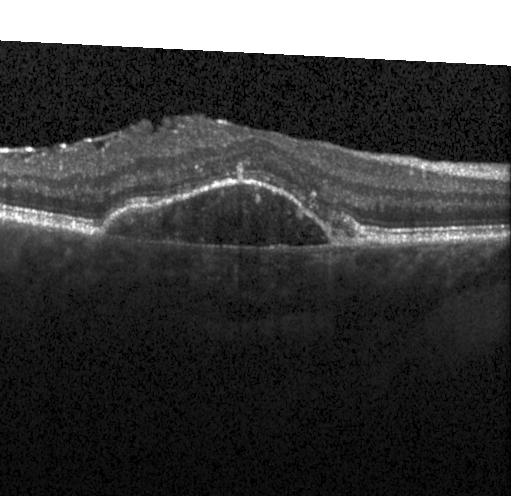
Heidelberg Spectralis OCT system. Optical coherence tomography scan. Horizontal scan through the fovea. SD-OCT.
Assessment: a choroidal neovascular membrane.